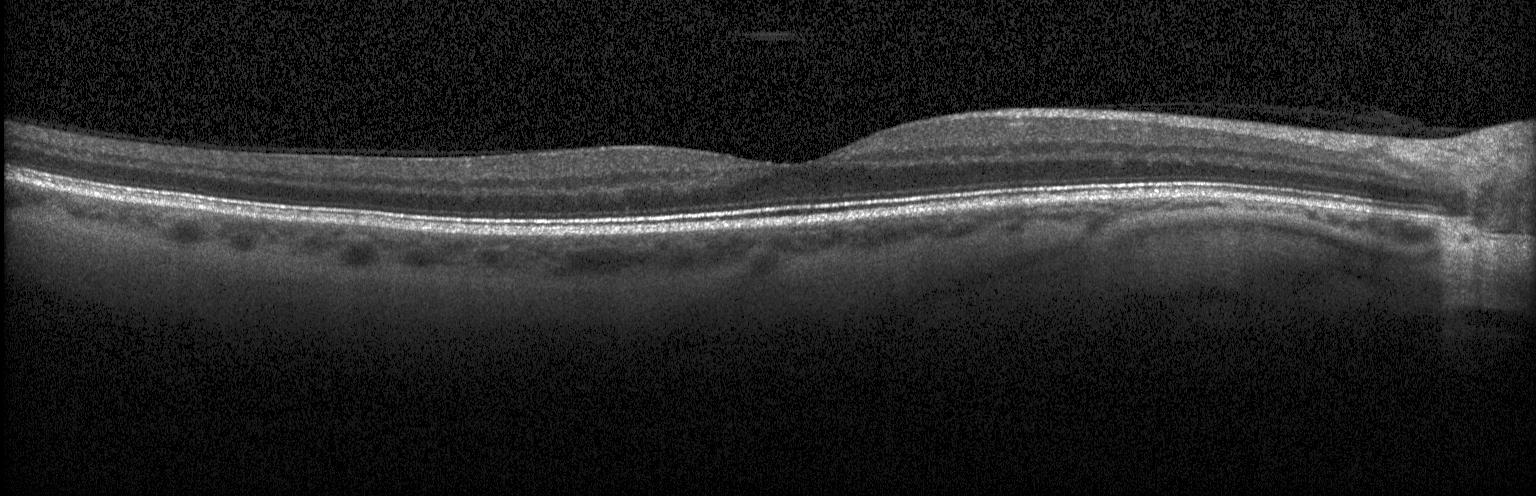
Spectral-domain OCT B-scan: neither CNV, DME, nor drusen.